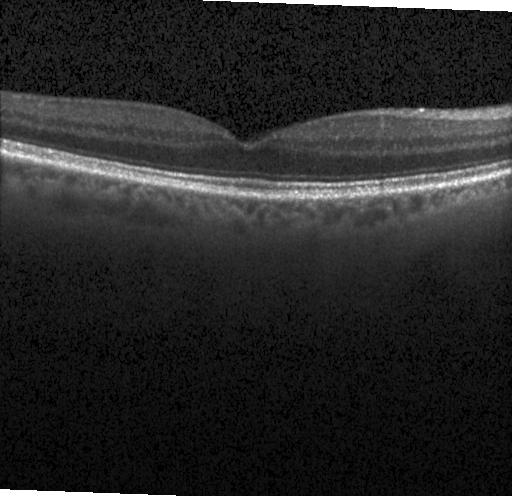

OCT B-scan
No CNV, no DME, and no drusen.